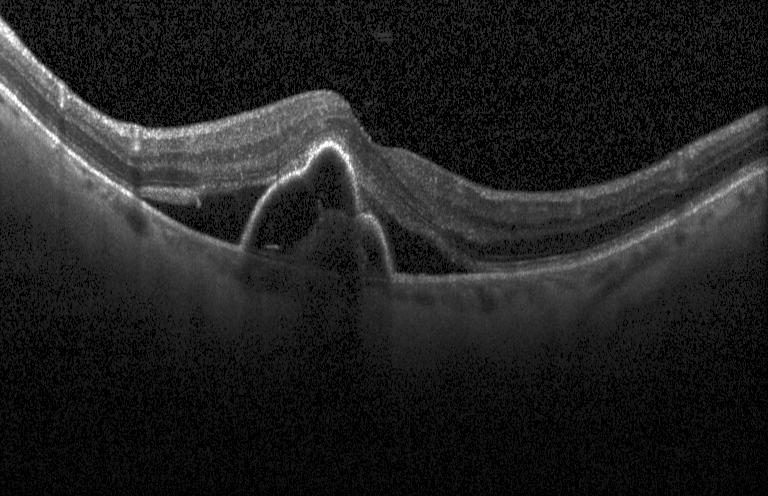

Retinal OCT cross-section showing choroidal neovascularization (CNV).